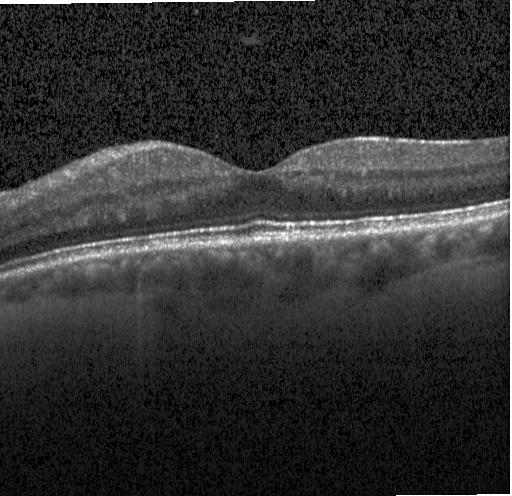

OCT B-scan showing no choroidal neovascularization, no diabetic macular edema, and no drusen.